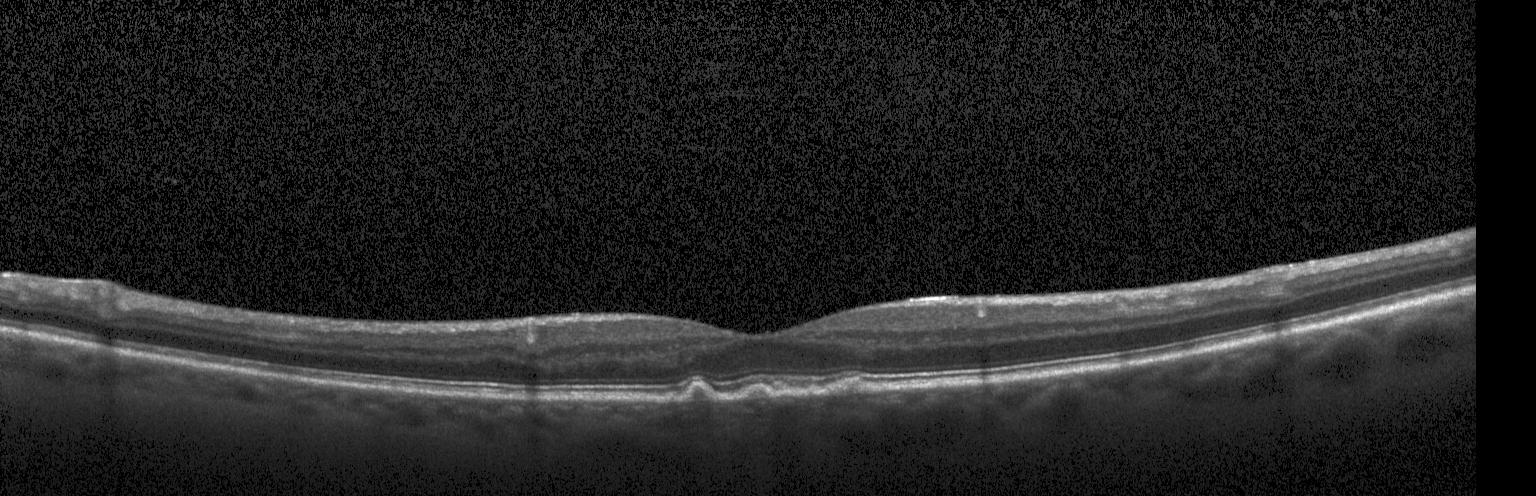

Horizontal scan through the fovea; instrument: Heidelberg Spectralis; OCT B-scan; SD-OCT — Dx: drusen.